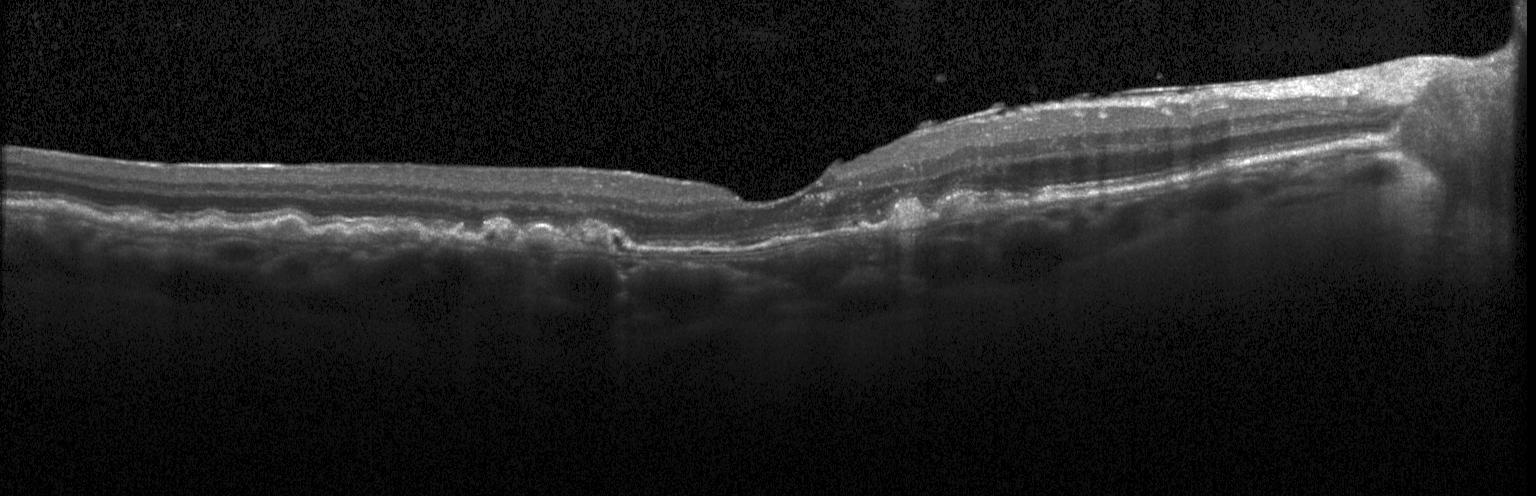
Retinal OCT cross-section. Macular scan.
Diagnosis: a choroidal neovascular membrane.